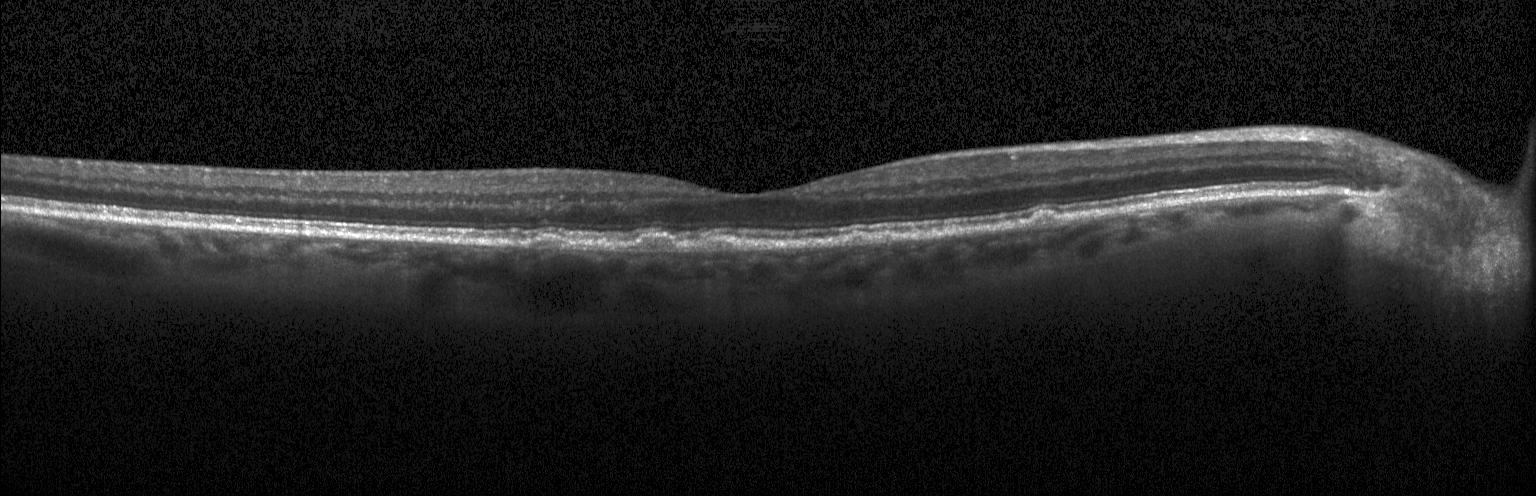
Macular scan, spectral-domain OCT, instrument: Heidelberg Spectralis, retinal OCT B-scan — Finding: drusen.